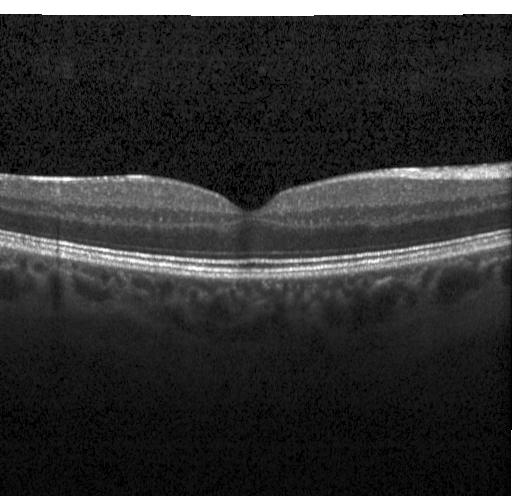 Instrument: Heidelberg Spectralis, optical coherence tomography scan
Finding: neither choroidal neovascularization, diabetic macular edema, nor drusen.